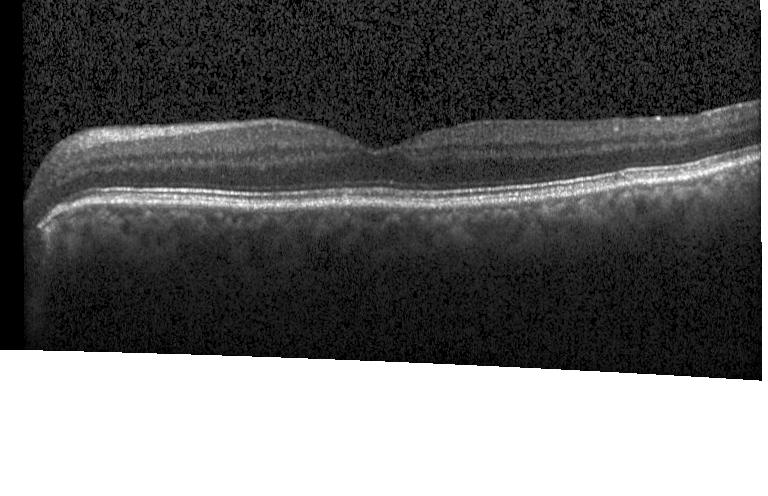

Impression: no choroidal neovascularization, diabetic macular edema, or drusen.